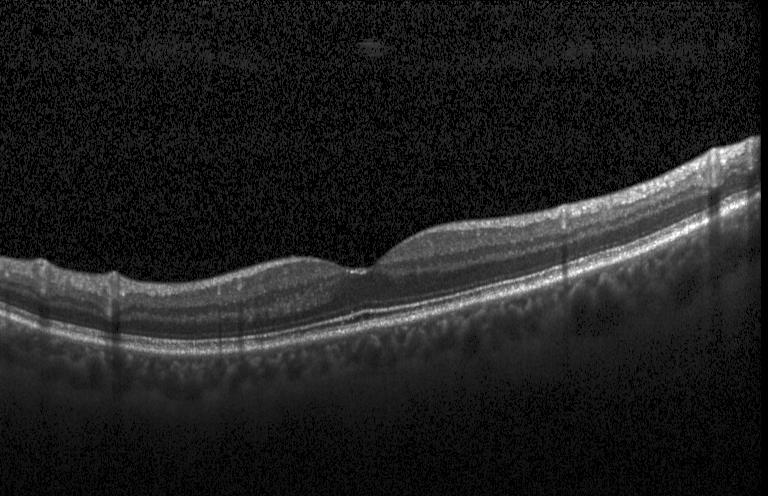

Spectral-domain optical coherence tomography; optical coherence tomography scan; through the macula; acquired on a Heidelberg Spectralis — Dx: no evidence of choroidal neovascularization, diabetic macular edema, or drusen.